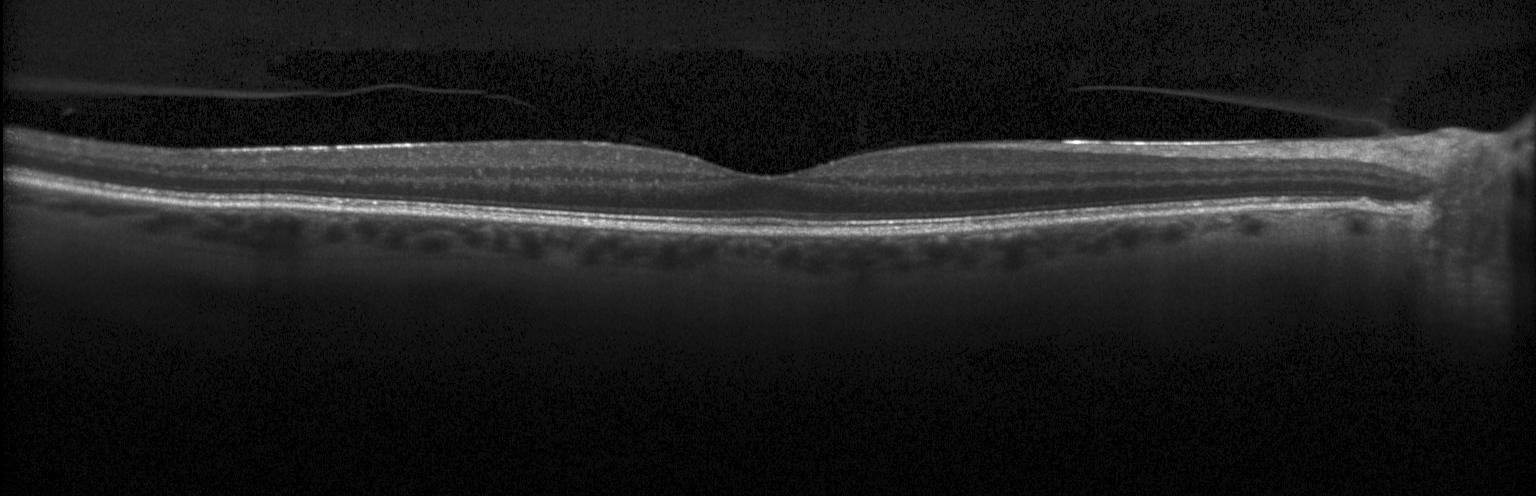 Heidelberg Spectralis OCT system. Through the macula. Retinal OCT cross-section. SD-OCT — Macular OCT: no choroidal neovascularization, diabetic macular edema, or drusen.